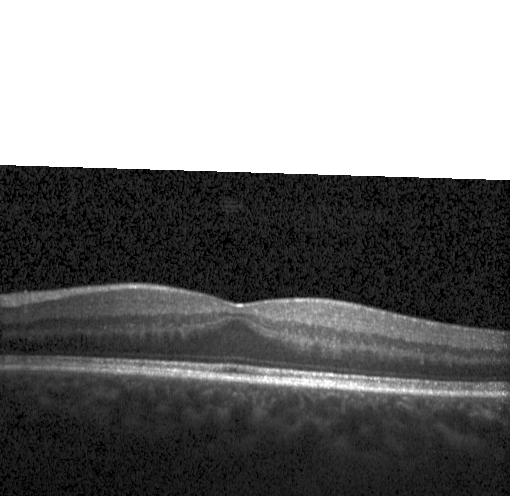 Retinal OCT cross-section showing no CNV, no DME, and no drusen.